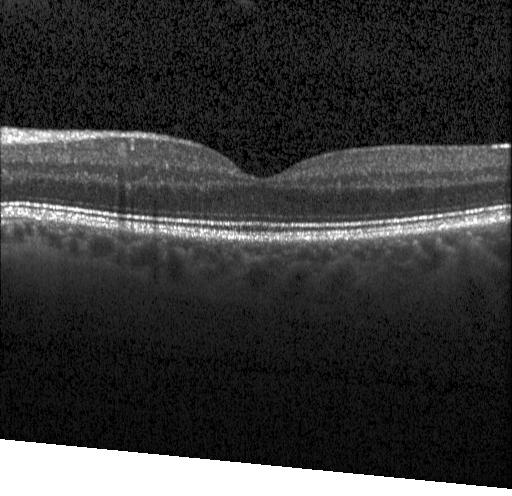

OCT B-scan — The scan shows neither CNV, DME, nor drusen.